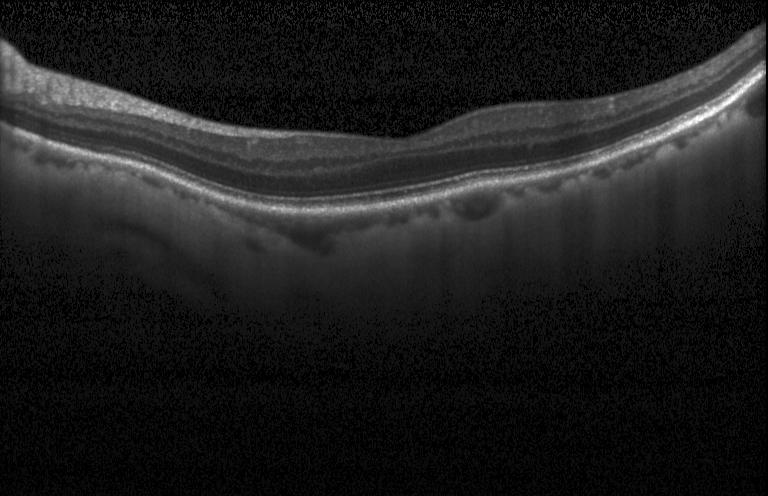 Optical coherence tomography scan.
Assessment: neither choroidal neovascularization, diabetic macular edema, nor drusen.